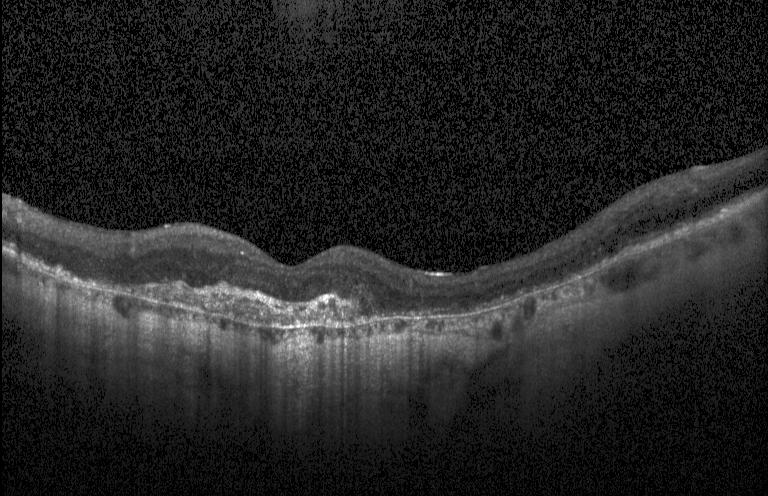 Impression: CNV.